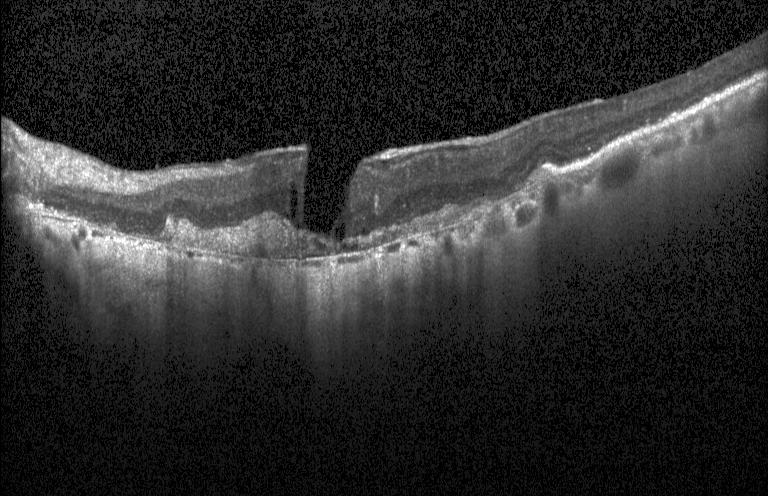

Acquired on a Heidelberg Spectralis · optical coherence tomography B-scan
This B-scan demonstrates choroidal neovascularization.